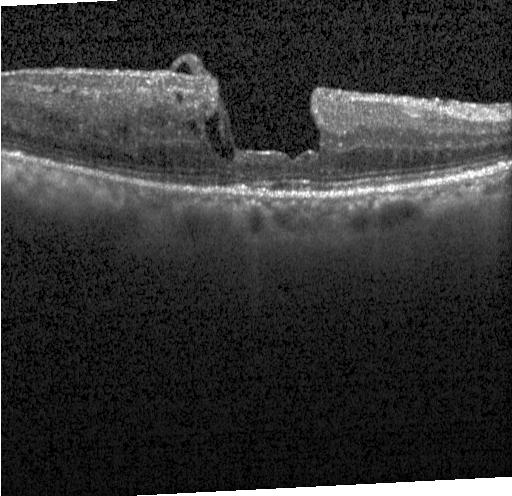

Macular OCT: diabetic macular edema (DME).